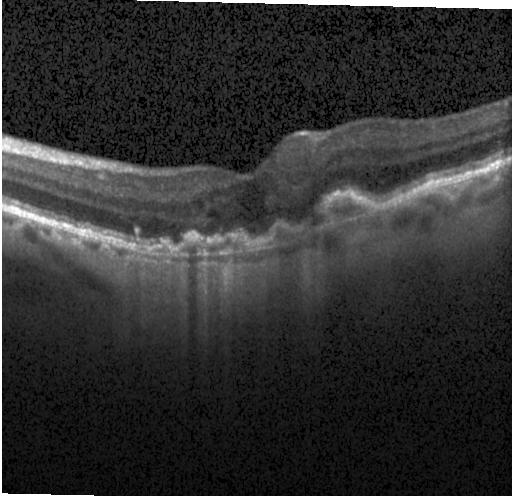
Impression: choroidal neovascularization.